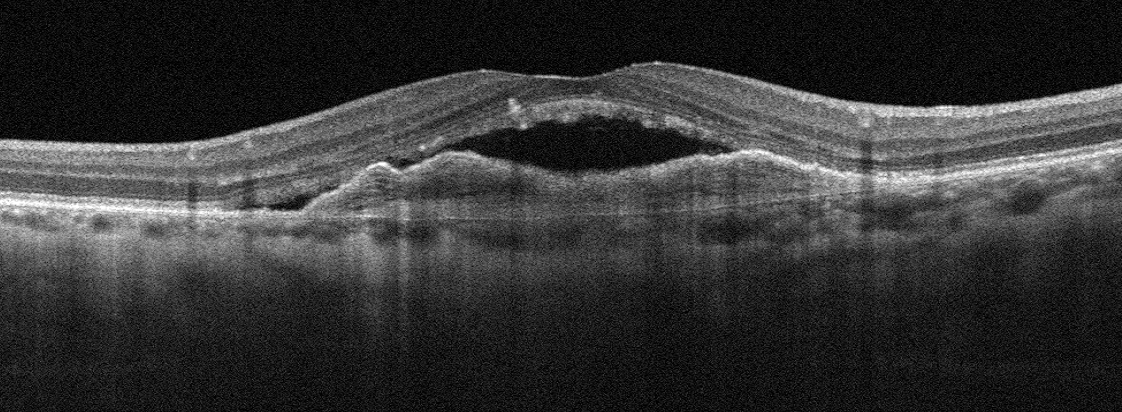
Instrument: Optovue Avanti RTVue XR · retinal OCT B-scan · fovea-centered.
This B-scan demonstrates age-related macular degeneration.